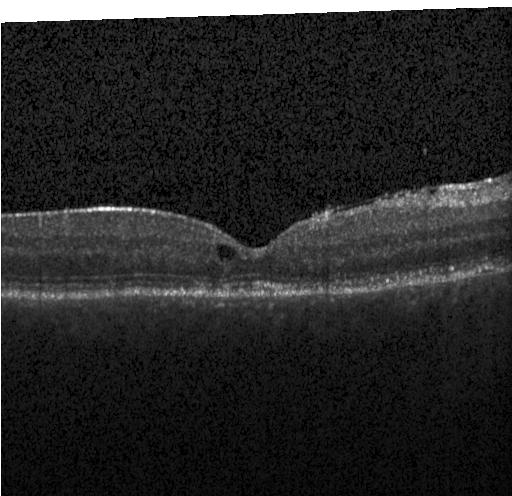

OCT finding: DME.